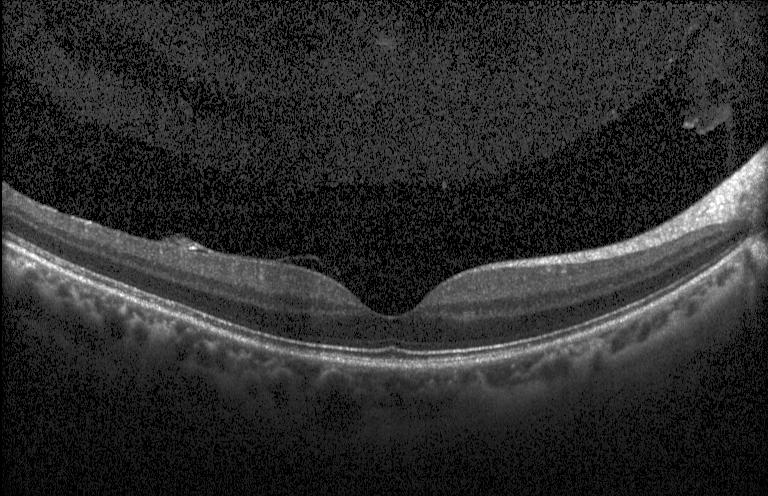
Macular scan · spectral-domain optical coherence tomography · OCT line scan. Finding: no choroidal neovascularization, diabetic macular edema, or drusen.